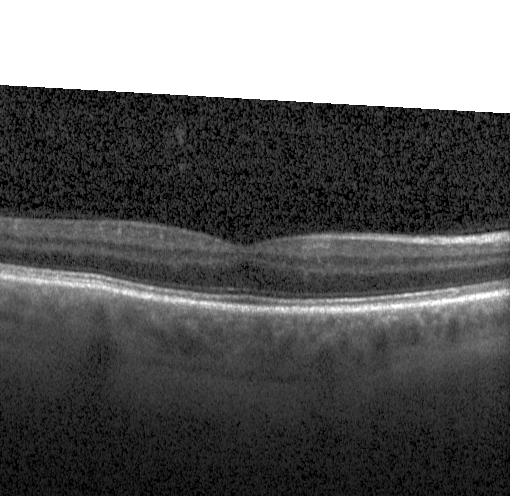
Retinal OCT B-scan; spectral-domain OCT; horizontal scan through the fovea; instrument: Heidelberg Spectralis. Impression: no evidence of choroidal neovascularization, diabetic macular edema, or drusen.